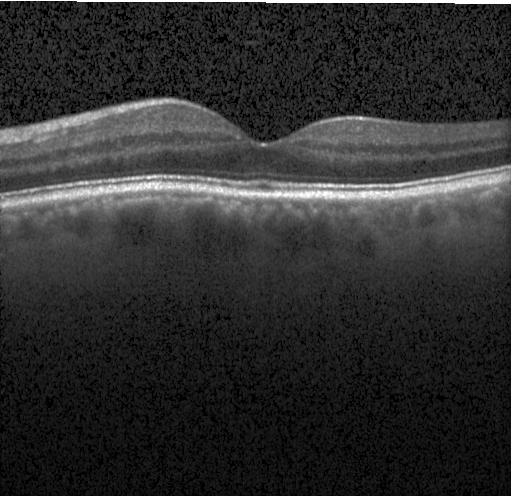 Optical coherence tomography scan; spectral-domain optical coherence tomography.
Finding: no CNV, DME, or drusen.